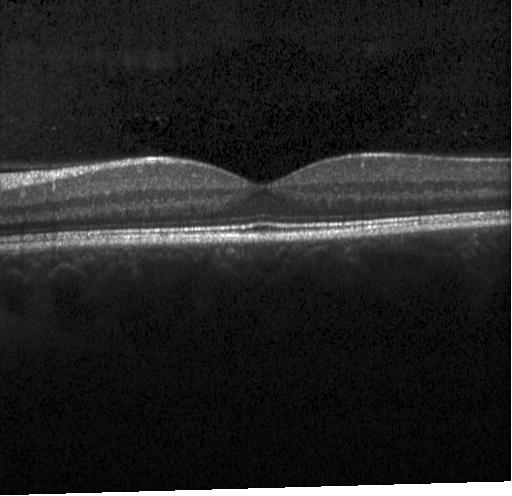 Spectral-domain OCT, horizontal scan through the fovea, retinal OCT B-scan, acquired on a Heidelberg Spectralis
No evidence of choroidal neovascularization, diabetic macular edema, or drusen.